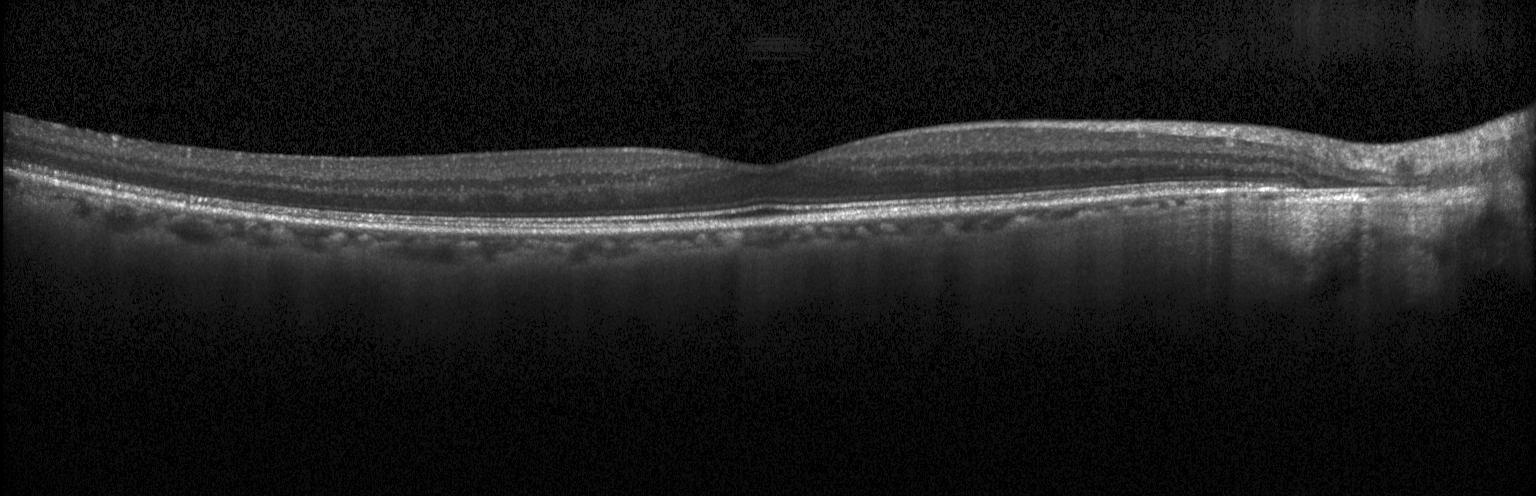 Impression: no evidence of choroidal neovascularization, diabetic macular edema, or drusen.